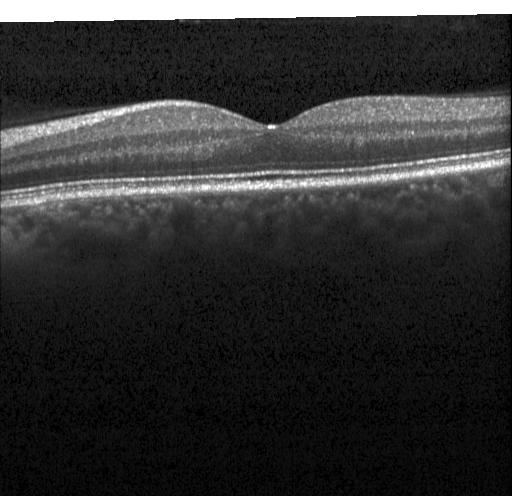

OCT line scan — Diagnosis: neither choroidal neovascularization, diabetic macular edema, nor drusen.